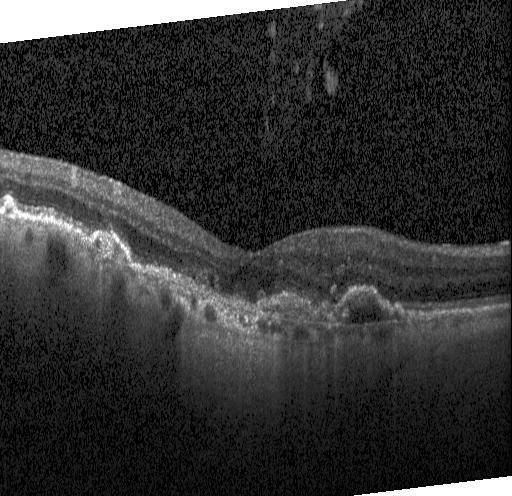

Spectral-domain OCT B-scan: a choroidal neovascular membrane.